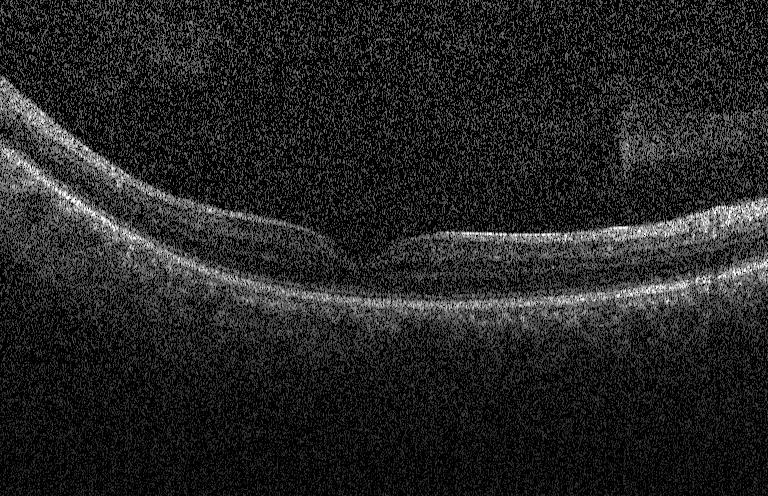
Retinal OCT cross-section — Finding: no evidence of CNV, DME, or drusen.